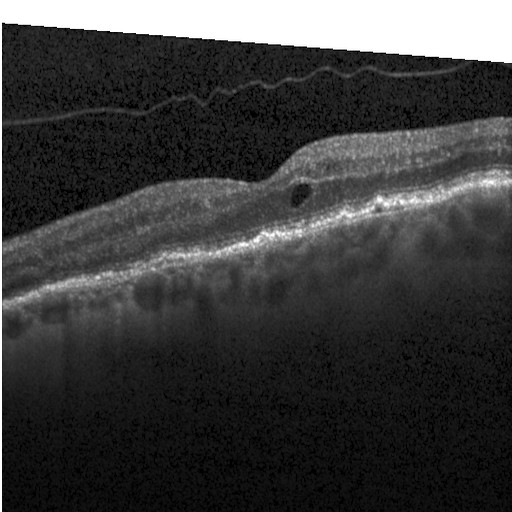

Diagnosis: diabetic macular edema (DME).